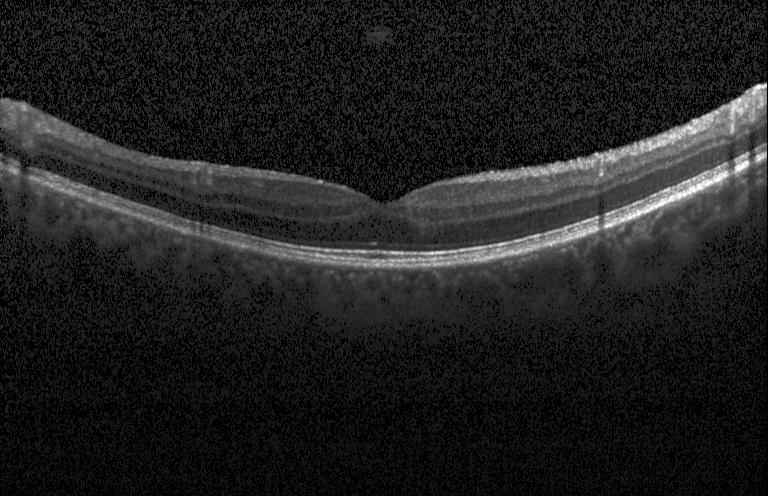

Finding: no CNV, DME, or drusen.